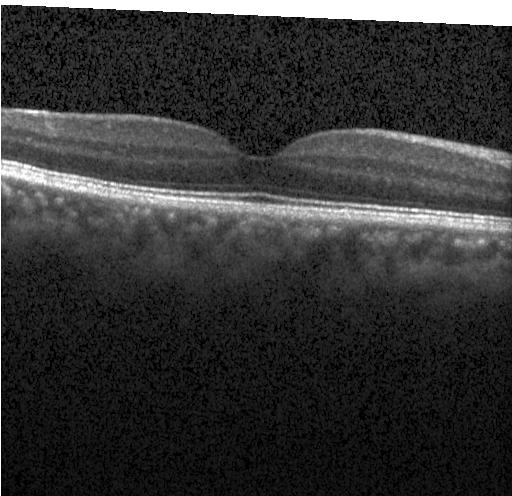 OCT line scan; spectral-domain OCT. This B-scan demonstrates no CNV, DME, or drusen.